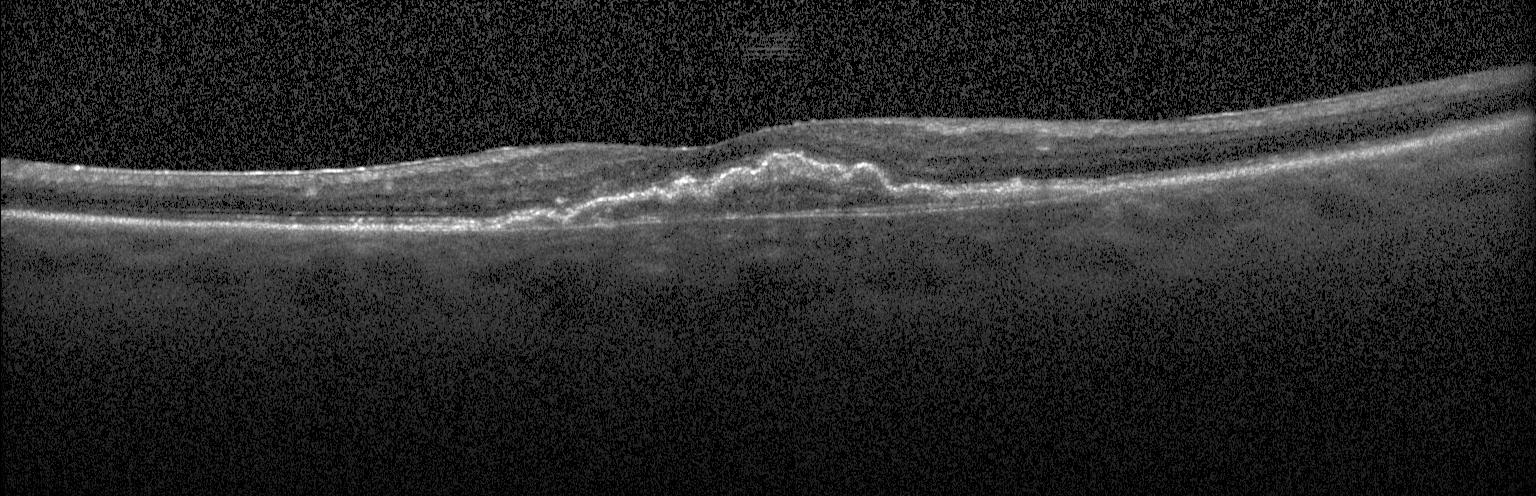

OCT line scan — Finding: choroidal neovascularization.